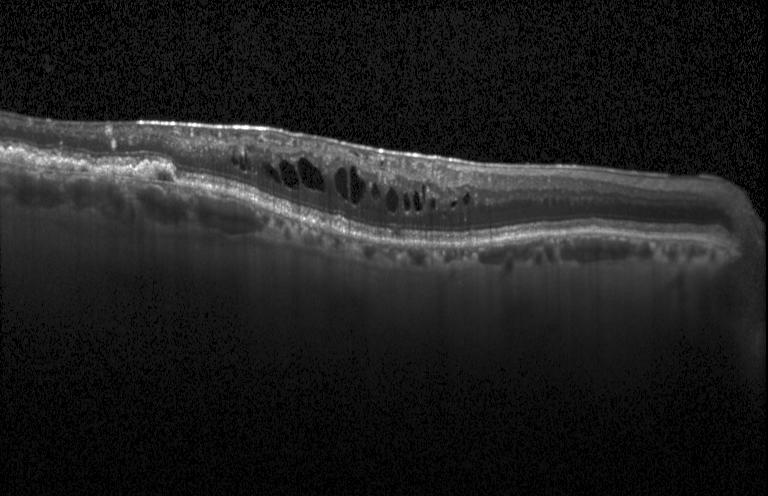

Heidelberg Spectralis; SD-OCT; retinal OCT B-scan. A choroidal neovascular membrane.